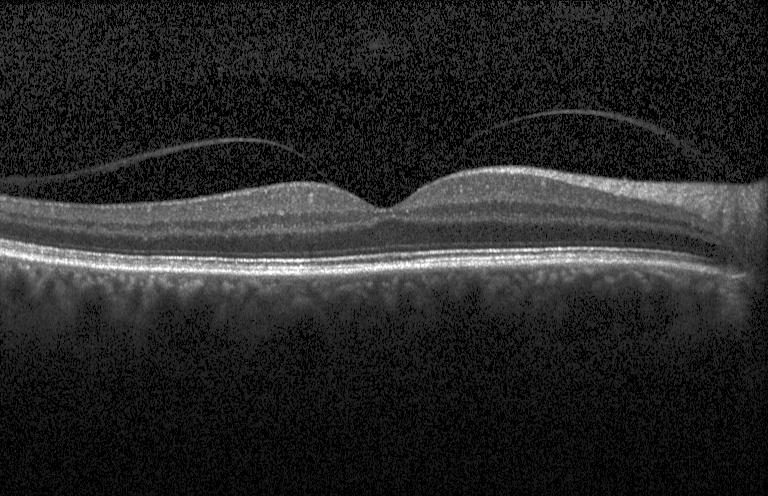 Retinal OCT B-scan — Impression: neither choroidal neovascularization, diabetic macular edema, nor drusen.